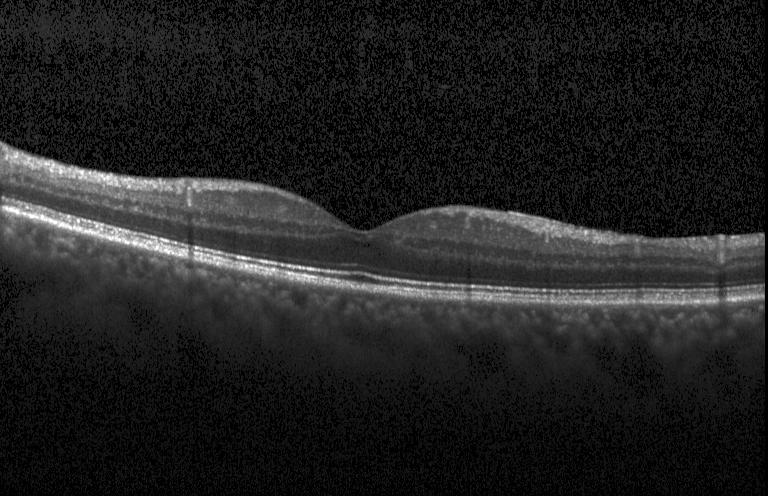 Dx: no choroidal neovascularization, diabetic macular edema, or drusen.